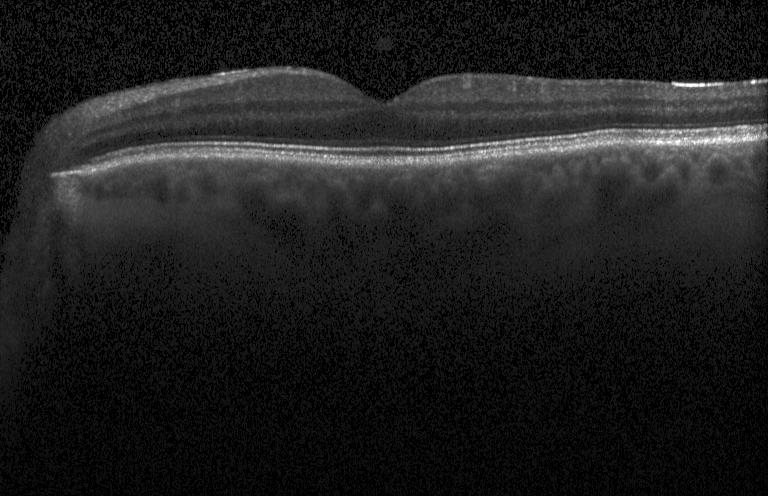
This B-scan demonstrates no CNV, DME, or drusen.